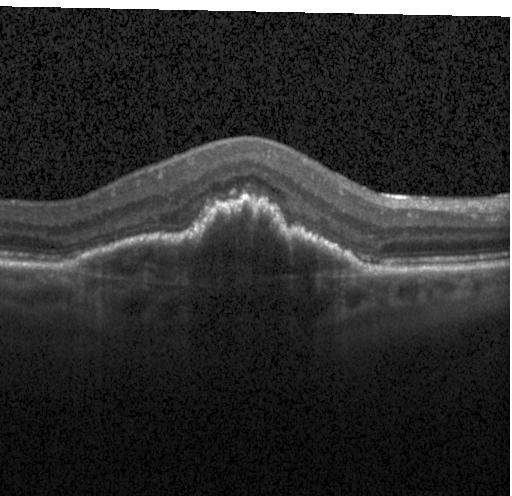 Through the macula. Optical coherence tomography scan. Spectral-domain optical coherence tomography. Assessment: a choroidal neovascular membrane.